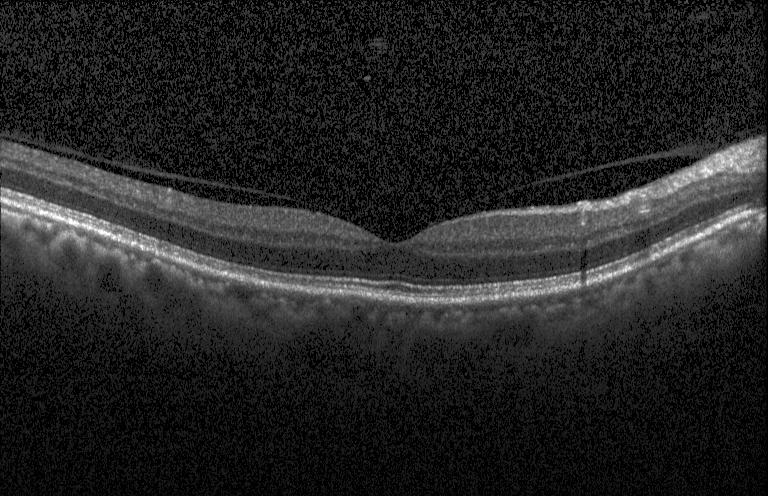

Spectral-domain OCT, retinal OCT B-scan, Heidelberg Spectralis — Neither CNV, DME, nor drusen.